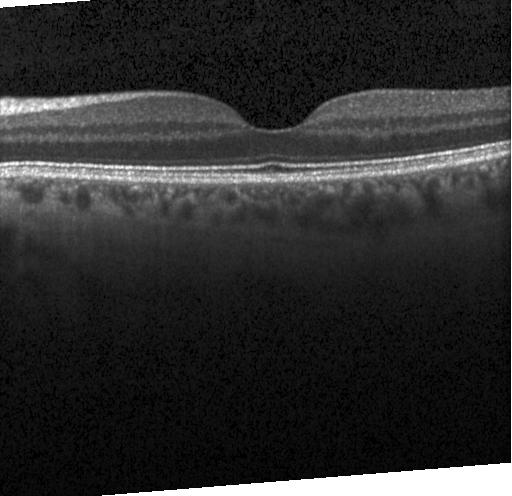

Acquired on a Heidelberg Spectralis, optical coherence tomography scan, spectral-domain optical coherence tomography.
Assessment: neither choroidal neovascularization, diabetic macular edema, nor drusen.